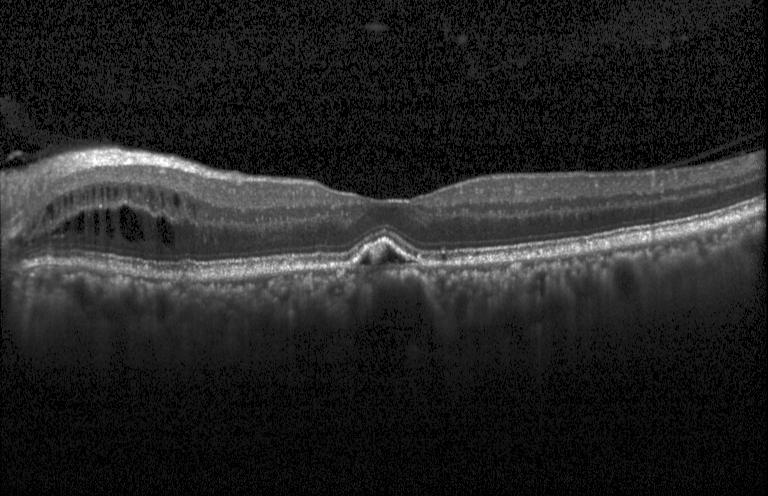
OCT B-scan; spectral-domain OCT
Finding: choroidal neovascularization.